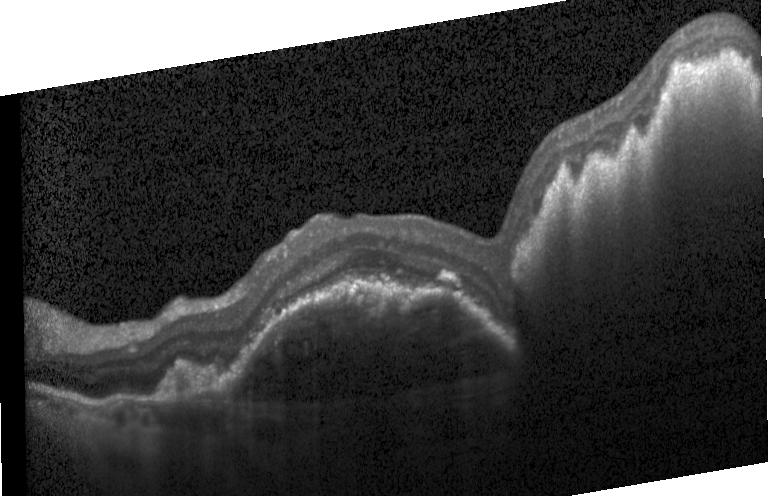
Impression: a choroidal neovascular membrane.